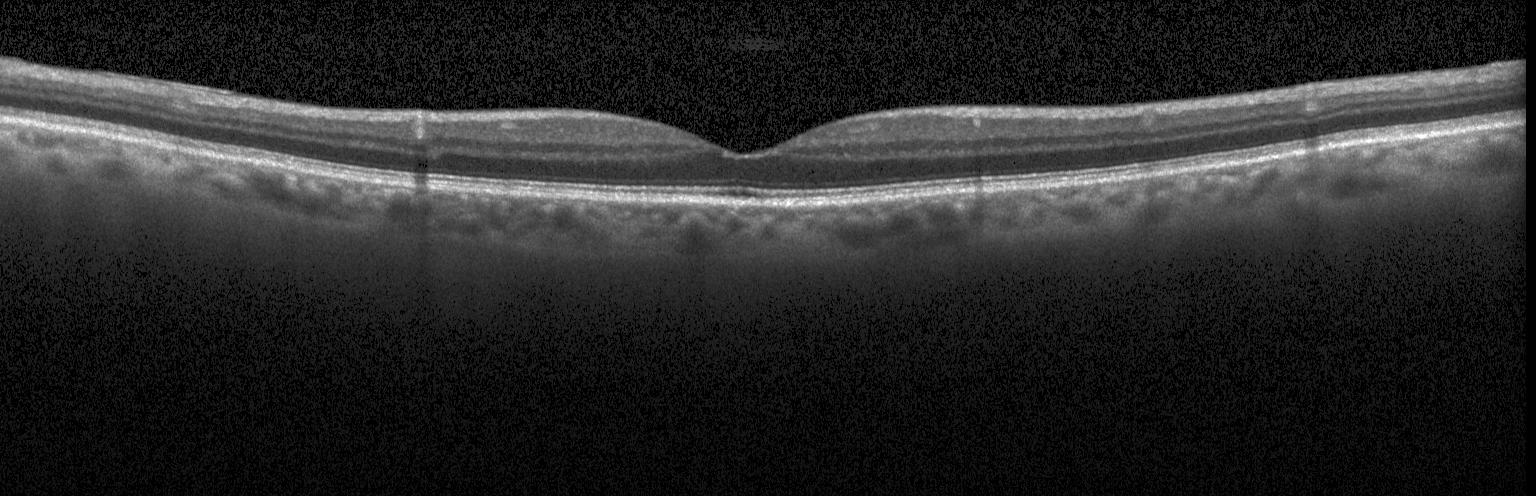 OCT line scan; spectral-domain optical coherence tomography. Impression: no choroidal neovascularization, diabetic macular edema, or drusen.